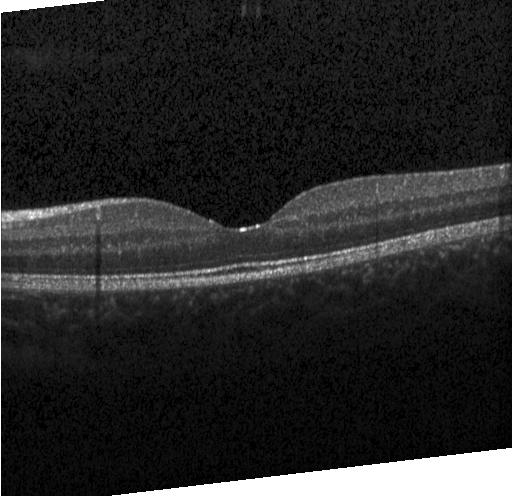
OCT scan showing no CNV, no DME, and no drusen.